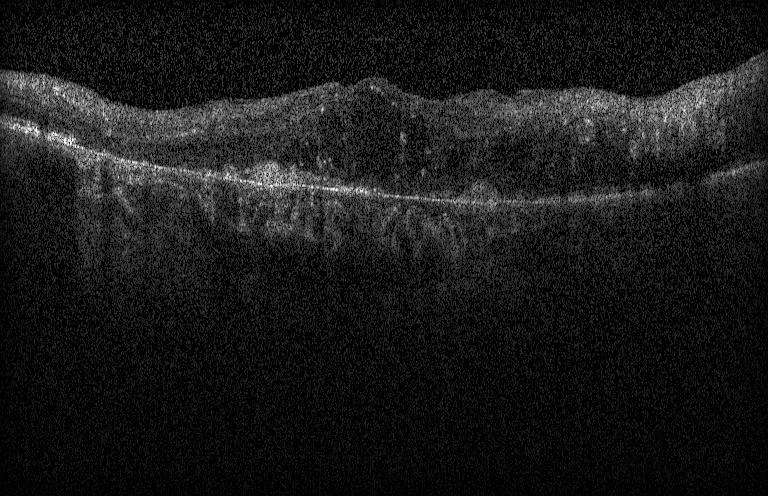

Retinal OCT B-scan, Heidelberg Spectralis OCT system, SD-OCT, macular scan. Impression: CNV.